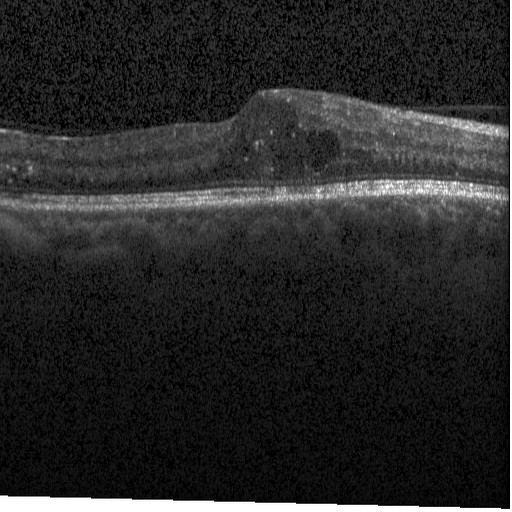

The scan shows diabetic macular edema (DME).